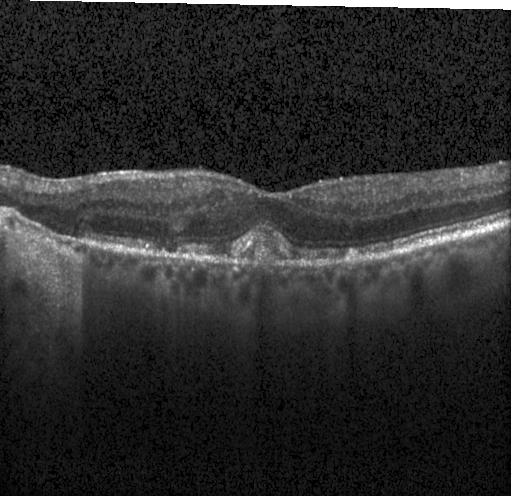
Macular OCT: a choroidal neovascular membrane.